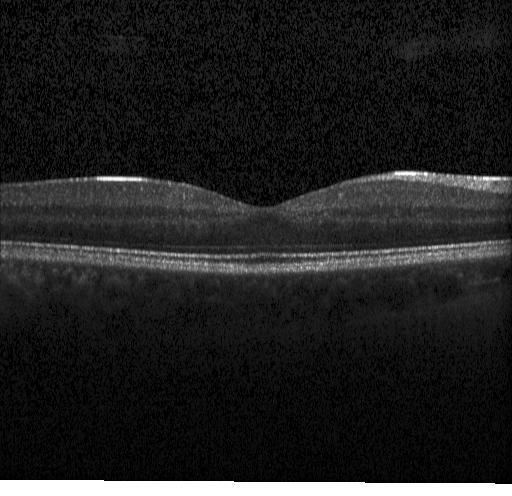
Spectral-domain optical coherence tomography; Heidelberg Spectralis; retinal OCT cross-section; fovea-centered
This B-scan demonstrates no choroidal neovascularization, no diabetic macular edema, and no drusen.